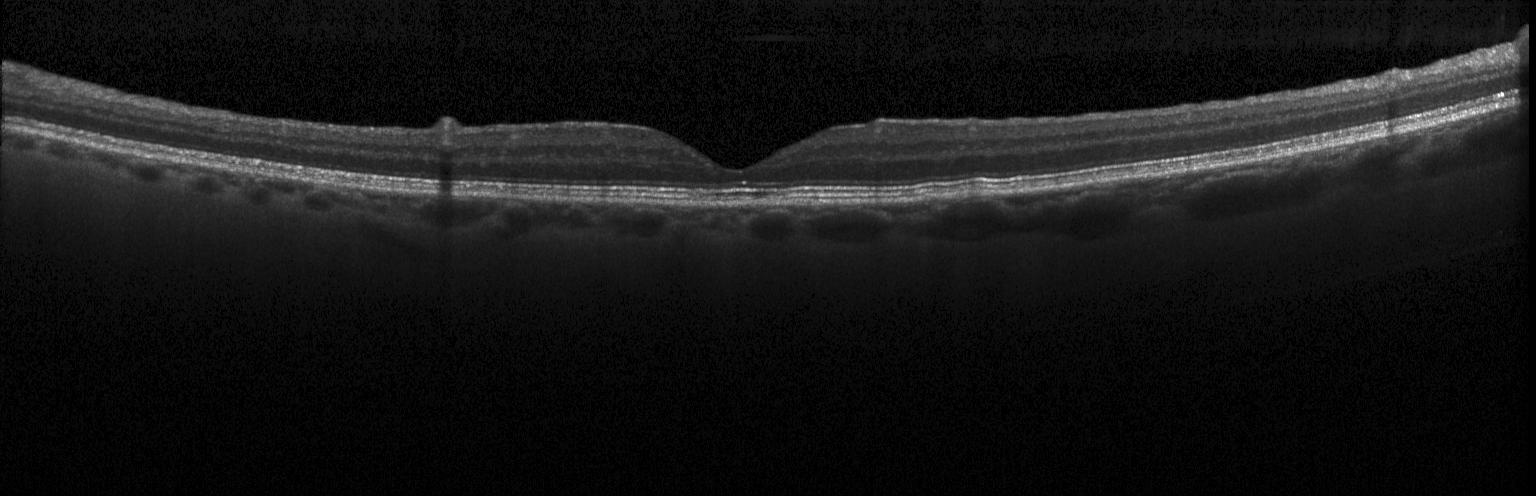
OCT line scan — Finding: neither CNV, DME, nor drusen.